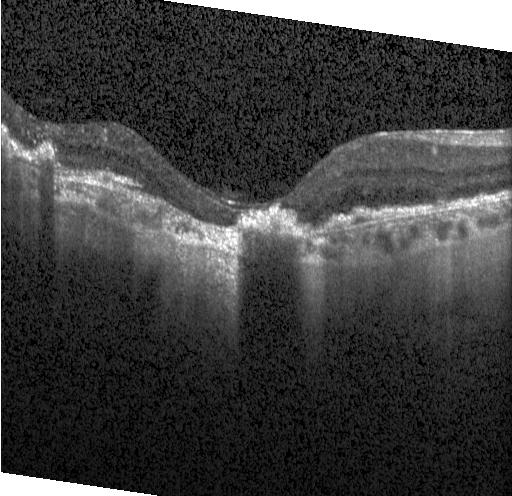

Retinal OCT B-scan, instrument: Heidelberg Spectralis, spectral-domain OCT. The scan shows choroidal neovascularization (CNV).